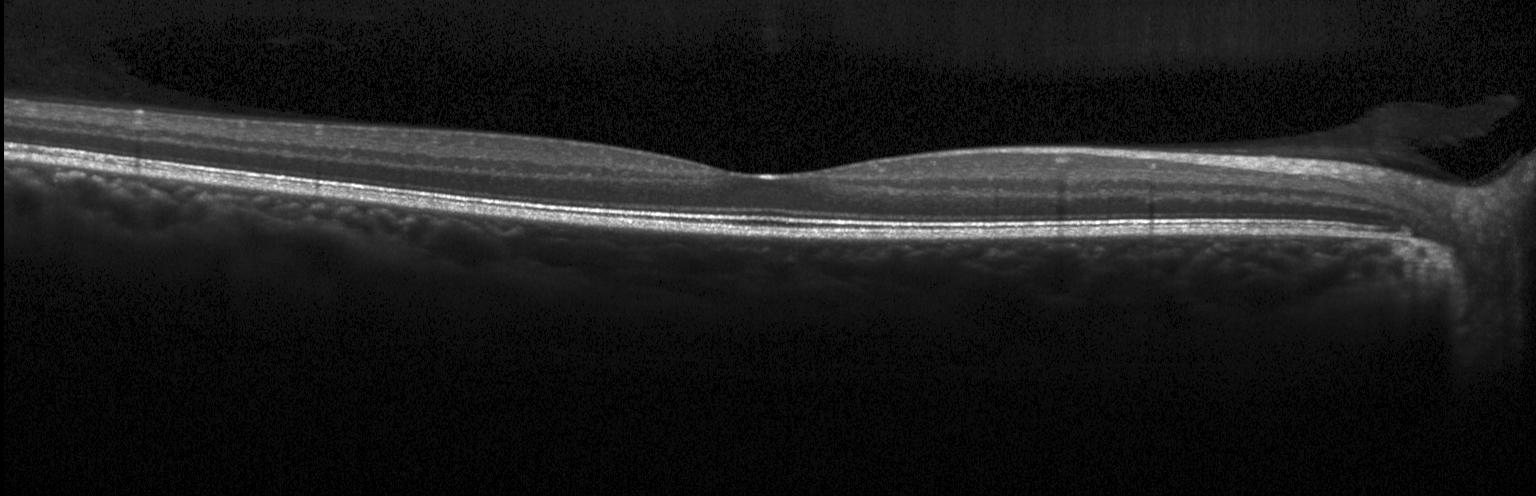

Retinal OCT B-scan · Heidelberg Spectralis — Diagnosis: neither choroidal neovascularization, diabetic macular edema, nor drusen.